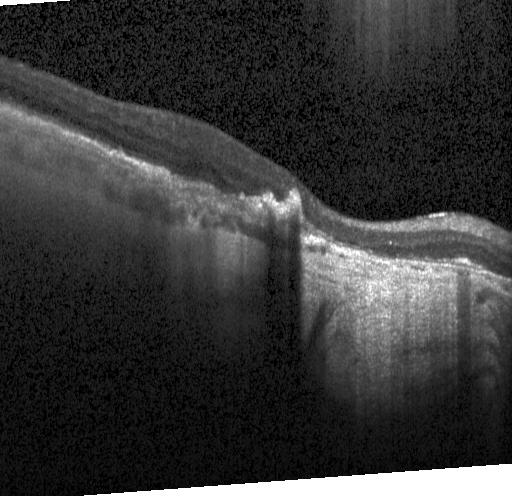

Optical coherence tomography scan. The scan shows choroidal neovascularization (CNV).